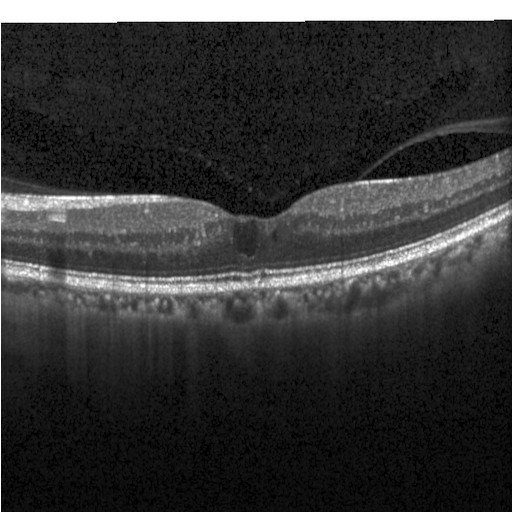
Retinal OCT cross-section; horizontal scan through the fovea. Finding: diabetic macular edema (DME).